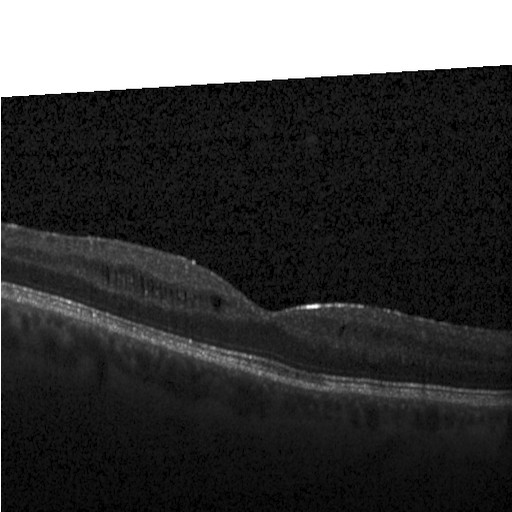

OCT B-scan.
Finding: DME.